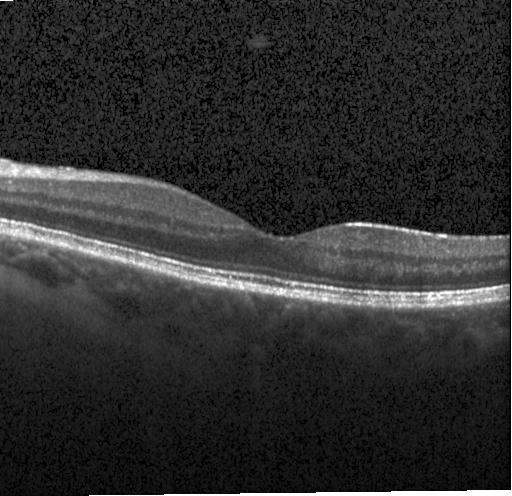
Diagnosis: no evidence of choroidal neovascularization, diabetic macular edema, or drusen.